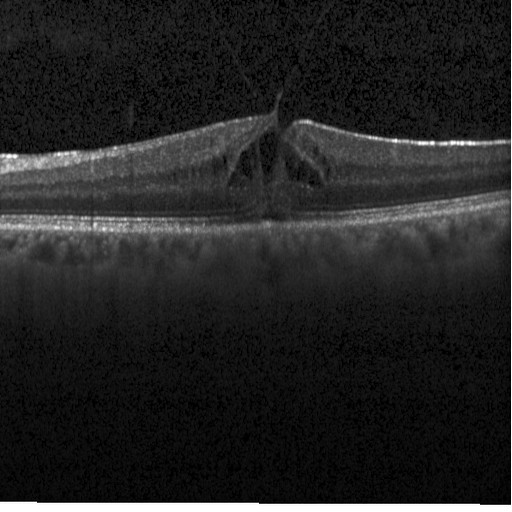 Acquired on a Heidelberg Spectralis, spectral-domain OCT, optical coherence tomography B-scan — Diagnosis: diabetic macular edema (DME).